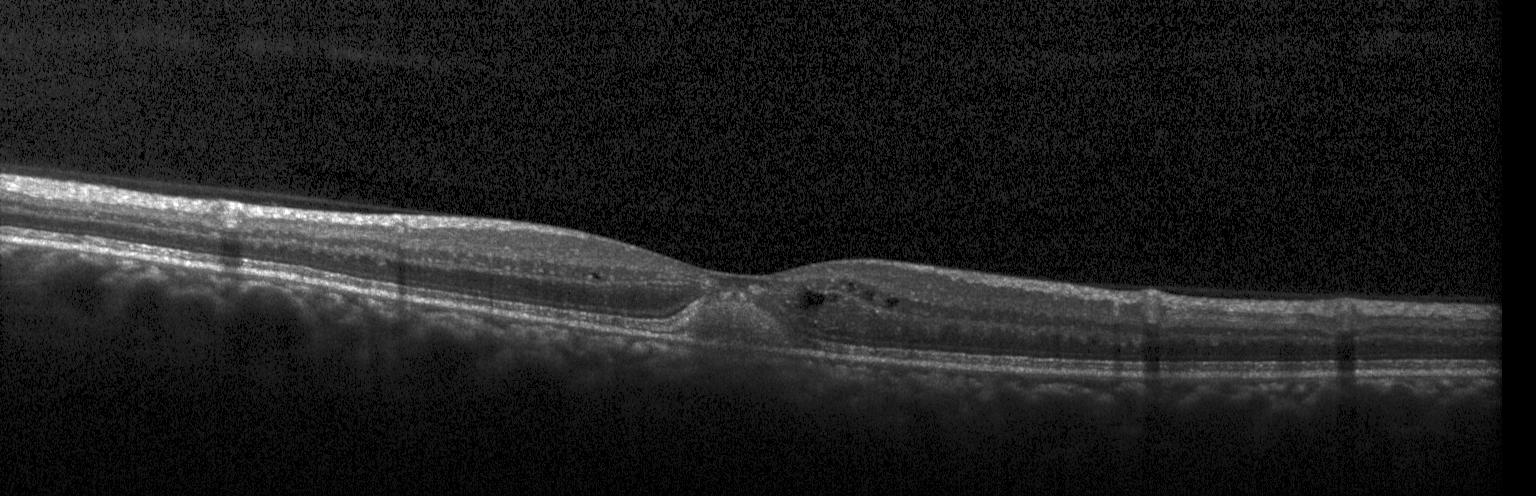

Finding: a choroidal neovascular membrane.